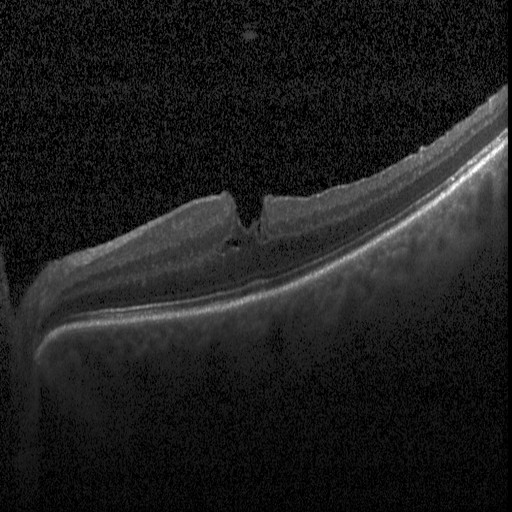

Diagnosis: DME.